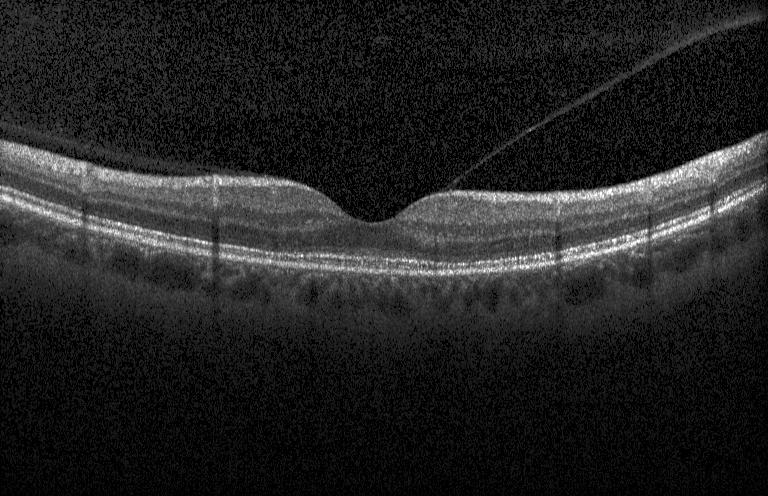 Diagnosis: neither choroidal neovascularization, diabetic macular edema, nor drusen.